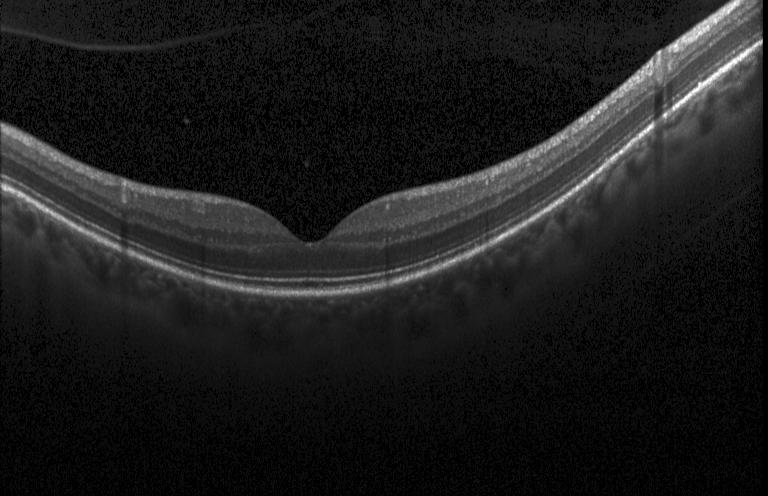 Through the macula. Retinal OCT B-scan. Heidelberg Spectralis. Spectral-domain OCT
OCT finding: neither choroidal neovascularization, diabetic macular edema, nor drusen.